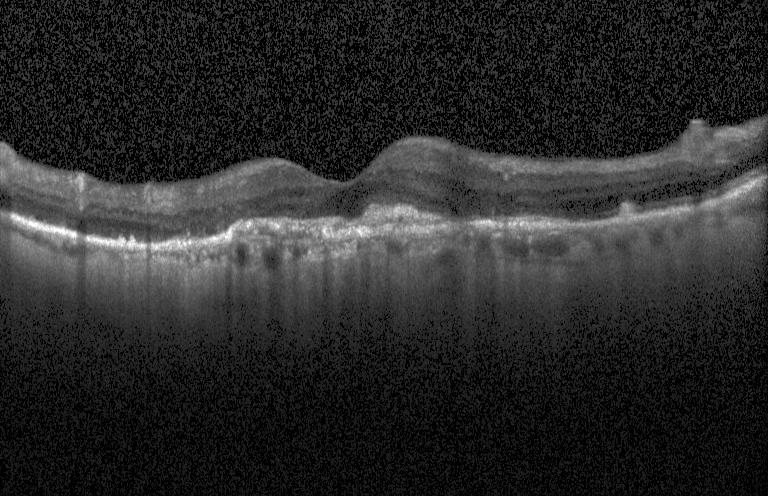 Macular OCT demonstrating CNV.